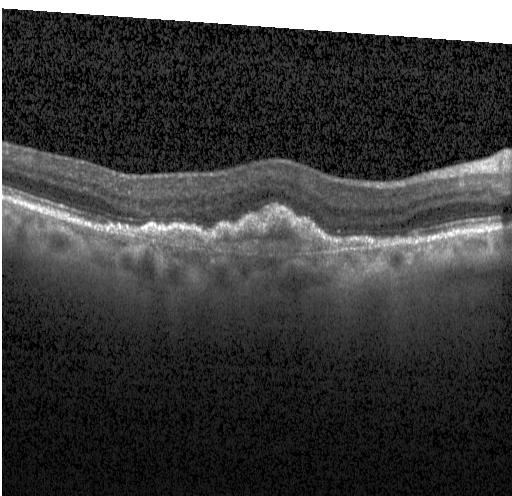

Spectral-domain OCT B-scan: a choroidal neovascular membrane.